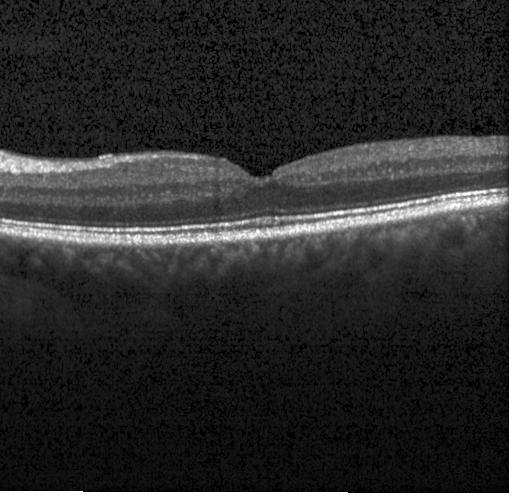

Through the macula · retinal OCT B-scan — The scan shows no CNV, no DME, and no drusen.